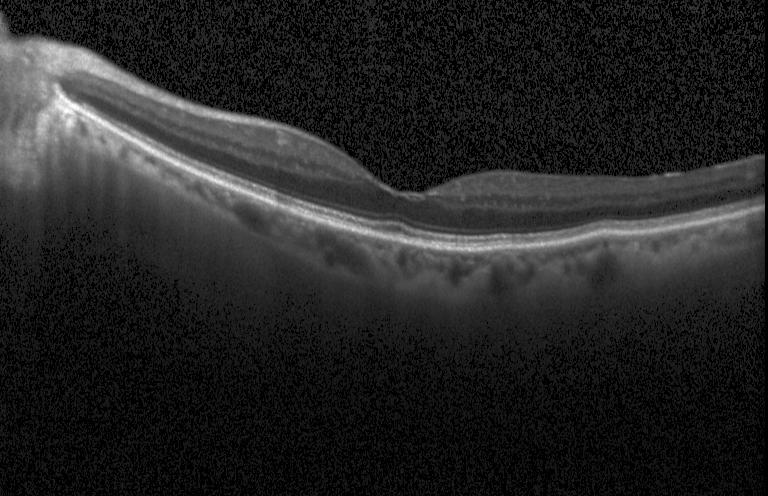 Retinal OCT cross-section showing no evidence of choroidal neovascularization, diabetic macular edema, or drusen.